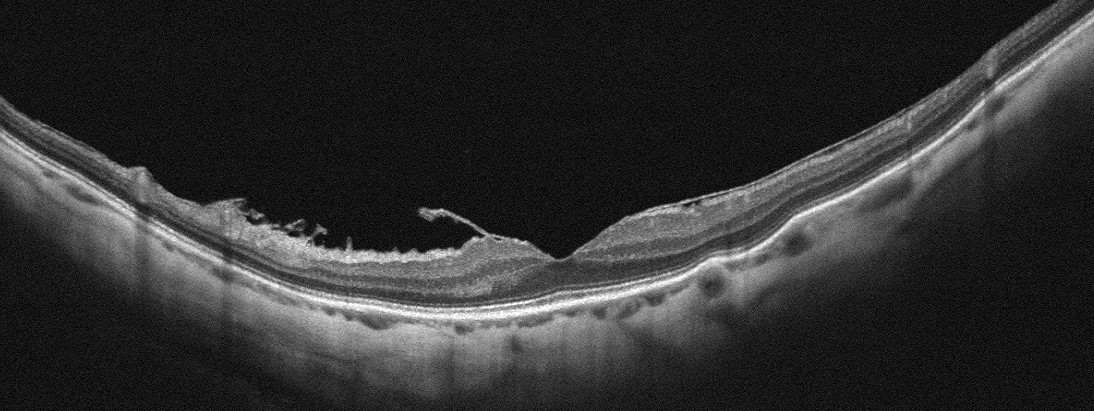
Fovea-centered, optical coherence tomography B-scan, instrument: Optovue Avanti RTVue XR. Impression: epiretinal membrane (ERM).